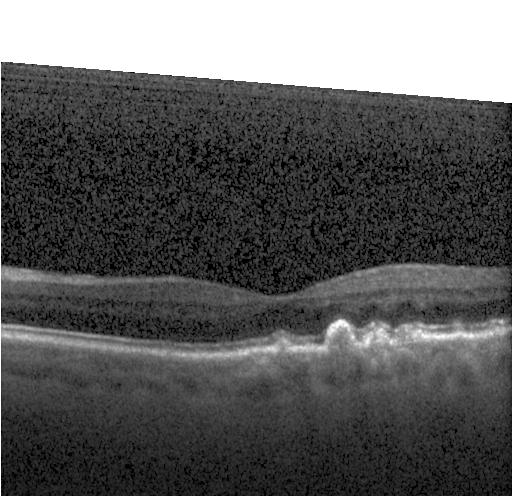
OCT B-scan; macular scan; acquired on a Heidelberg Spectralis; SD-OCT — Drusen.